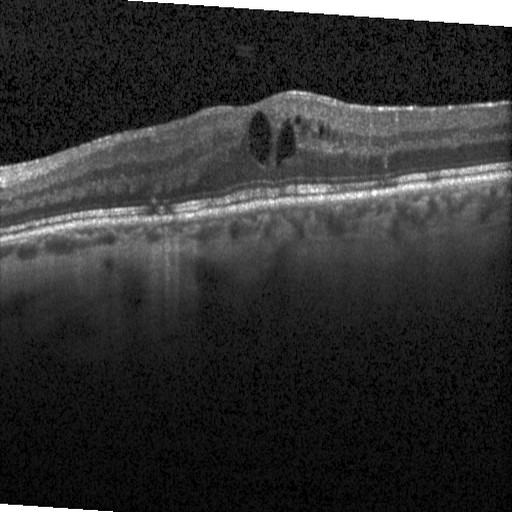
OCT line scan · macular scan. Finding: diabetic macular edema (DME).